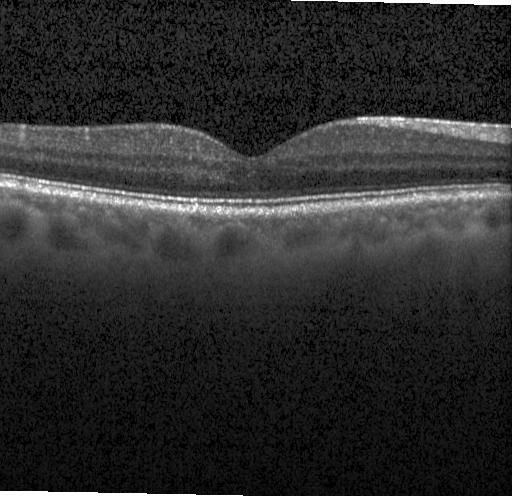 Heidelberg Spectralis OCT system · optical coherence tomography B-scan — Finding: no evidence of choroidal neovascularization, diabetic macular edema, or drusen.